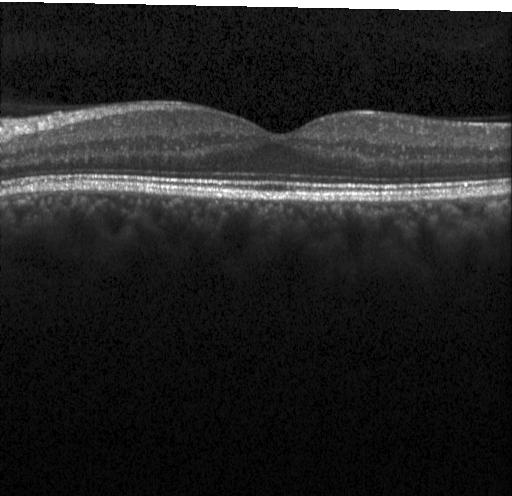
Impression: no choroidal neovascularization, diabetic macular edema, or drusen.